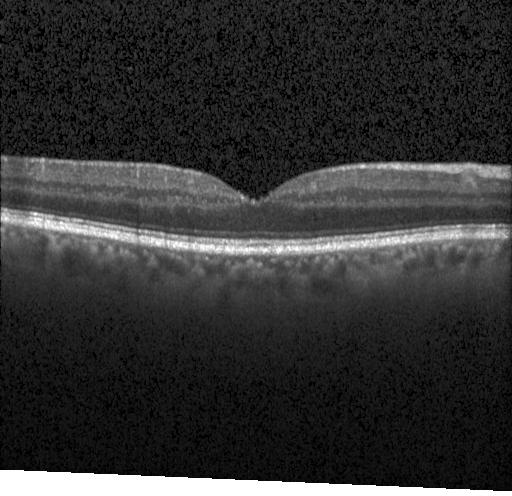

Fovea-centered; optical coherence tomography B-scan; SD-OCT.
Dx: neither choroidal neovascularization, diabetic macular edema, nor drusen.